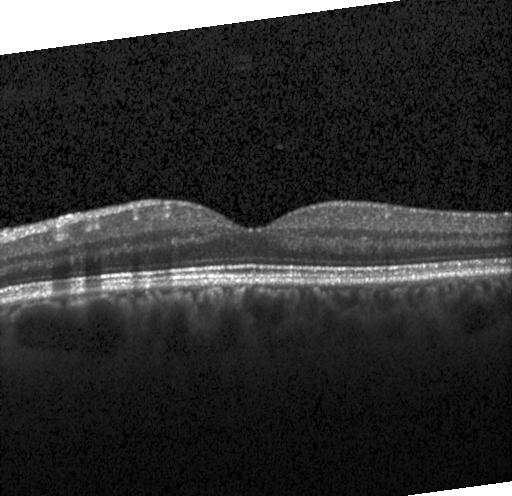 OCT B-scan
Finding: no evidence of choroidal neovascularization, diabetic macular edema, or drusen.